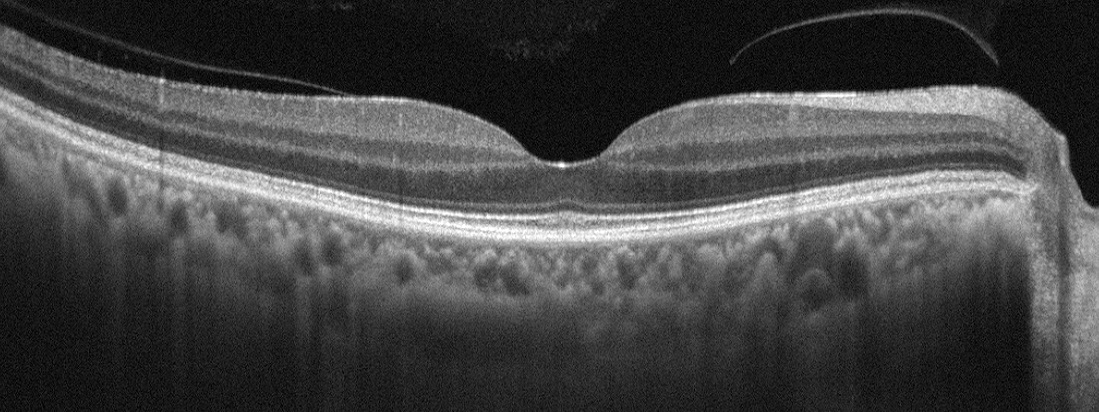 Diagnosis: ERM.